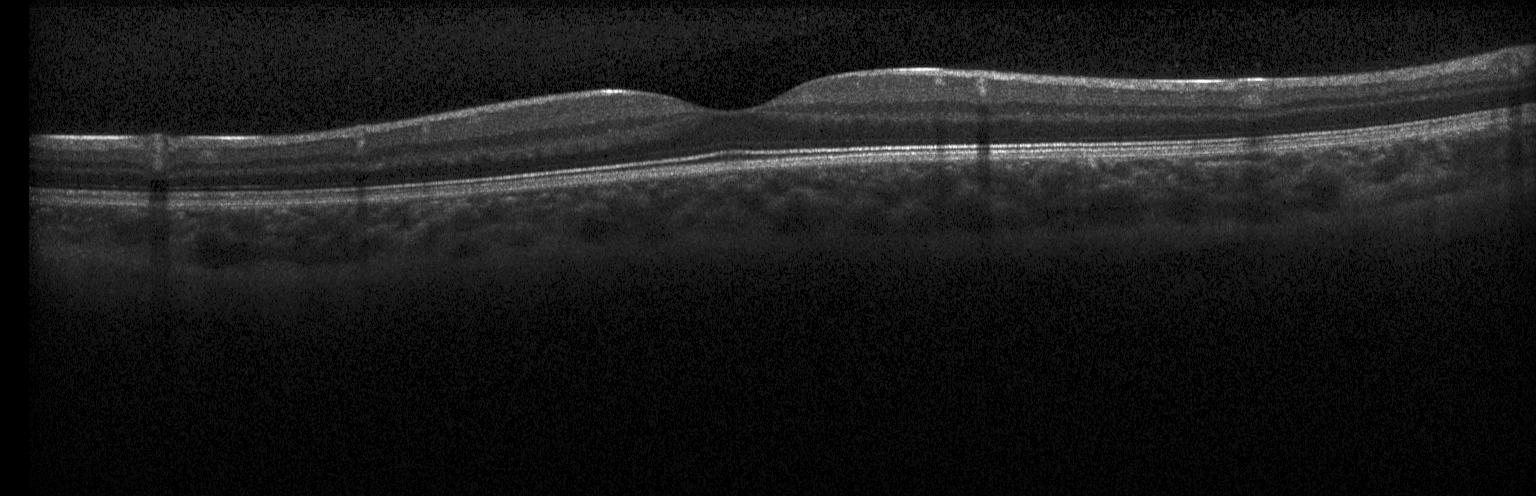
Diagnosis: no evidence of choroidal neovascularization, diabetic macular edema, or drusen.